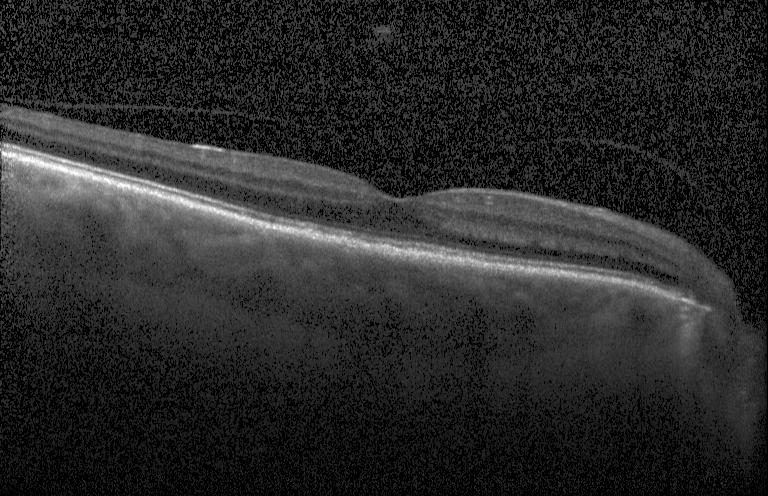
Heidelberg Spectralis. Fovea-centered. Spectral-domain optical coherence tomography. Optical coherence tomography B-scan
Macular OCT: no CNV, no DME, and no drusen.